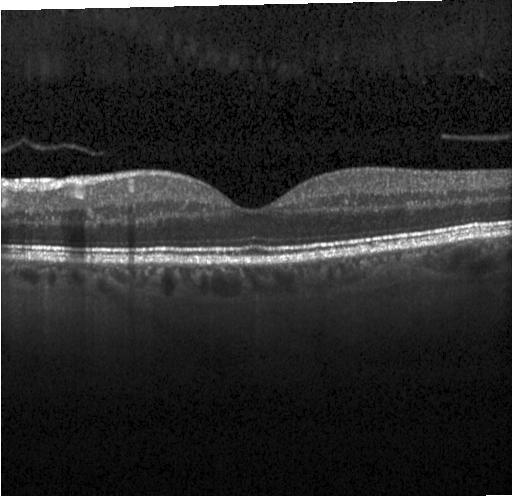 Spectral-domain OCT B-scan: no choroidal neovascularization, diabetic macular edema, or drusen.